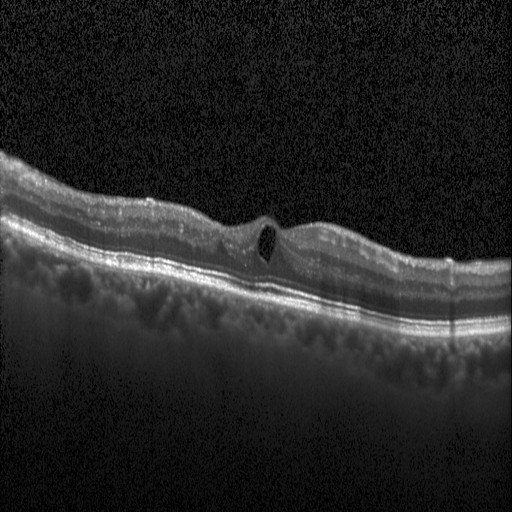
Retinal OCT cross-section showing DME.